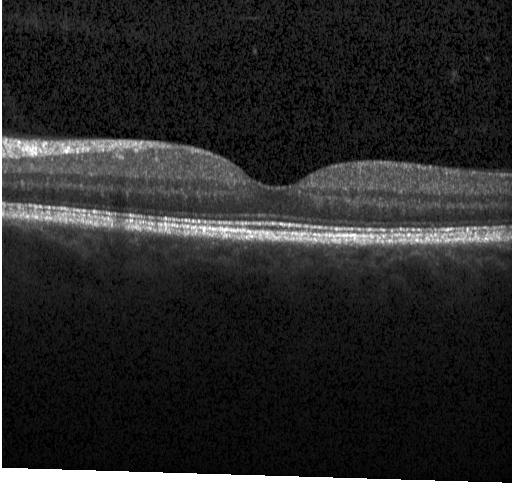

Retinal OCT cross-section. Heidelberg Spectralis. Fovea-centered — Assessment: neither CNV, DME, nor drusen.